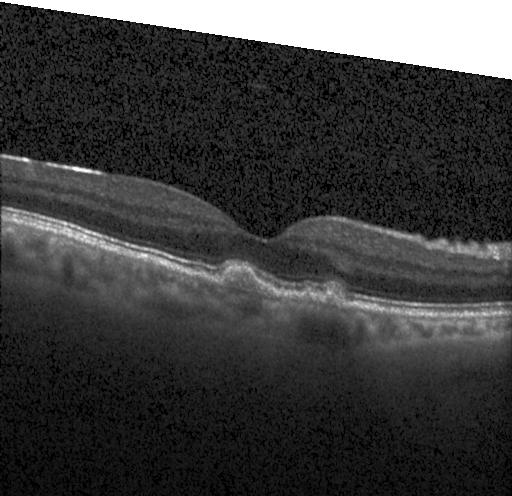 OCT finding: drusen.